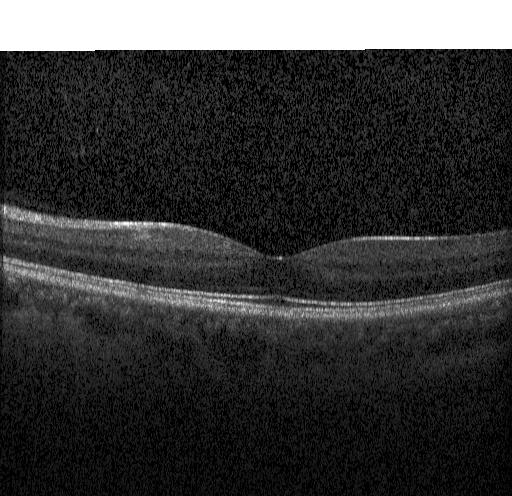
Optical coherence tomography B-scan; SD-OCT; horizontal scan through the fovea; instrument: Heidelberg Spectralis — No evidence of choroidal neovascularization, diabetic macular edema, or drusen.